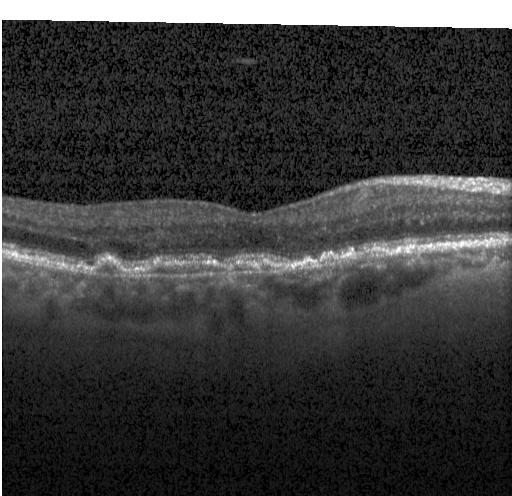 Fovea-centered. SD-OCT. Acquired on a Heidelberg Spectralis. Retinal OCT B-scan.
Diagnosis: CNV.